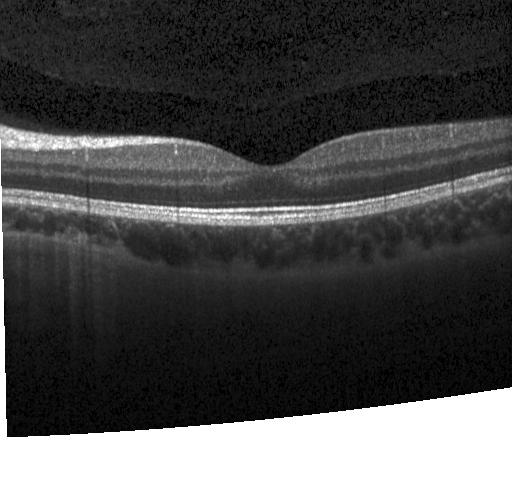
Neither CNV, DME, nor drusen.